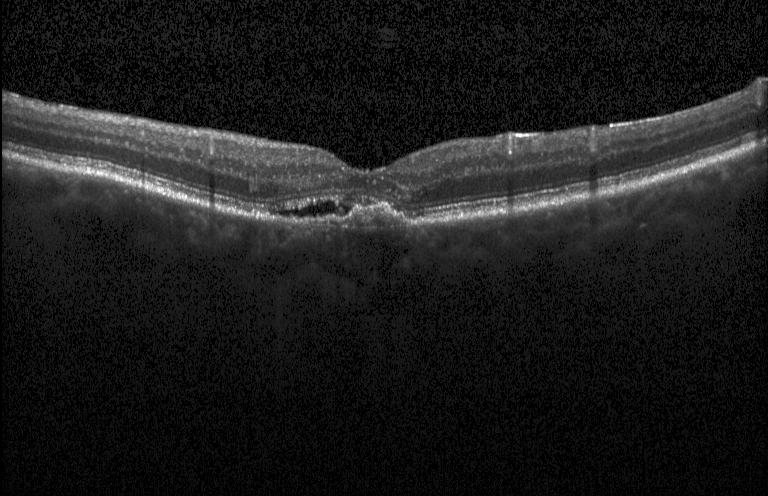
Retinal OCT cross-section.
Finding: a choroidal neovascular membrane.